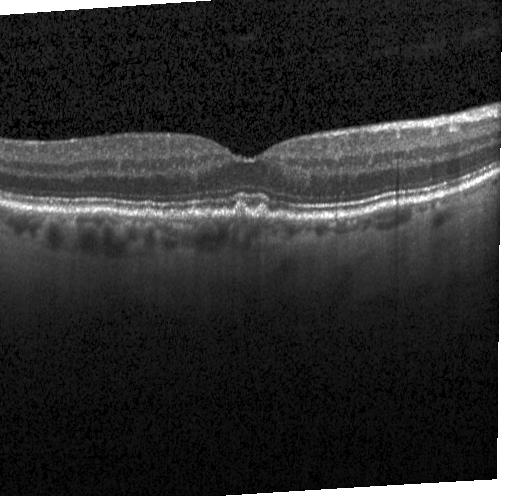
Impression: drusen.